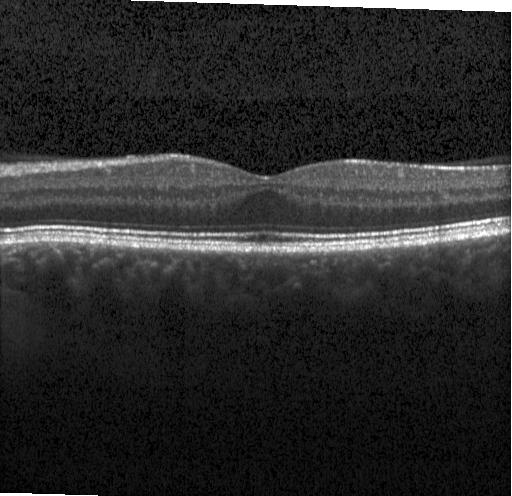

Finding: neither choroidal neovascularization, diabetic macular edema, nor drusen.